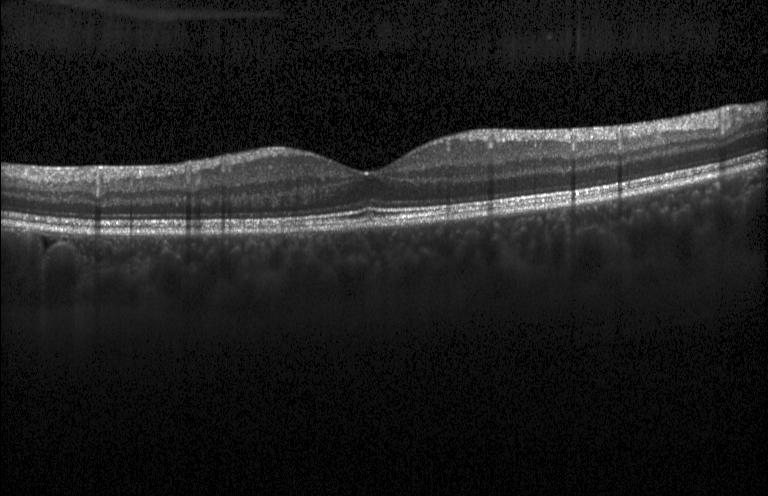
Centered on the fovea; spectral-domain optical coherence tomography; optical coherence tomography B-scan; instrument: Heidelberg Spectralis. Finding: neither choroidal neovascularization, diabetic macular edema, nor drusen.